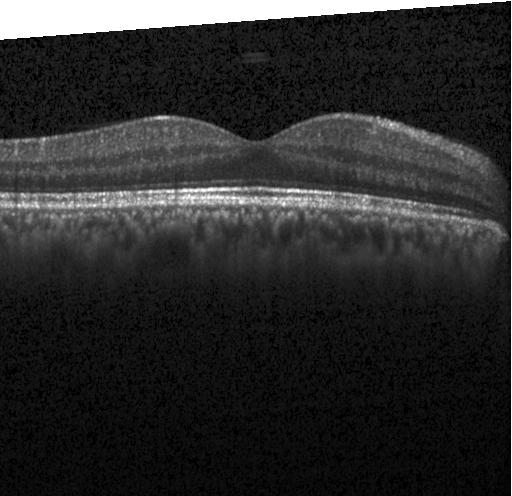
Retinal OCT cross-section · instrument: Heidelberg Spectralis
The scan shows no choroidal neovascularization, no diabetic macular edema, and no drusen.